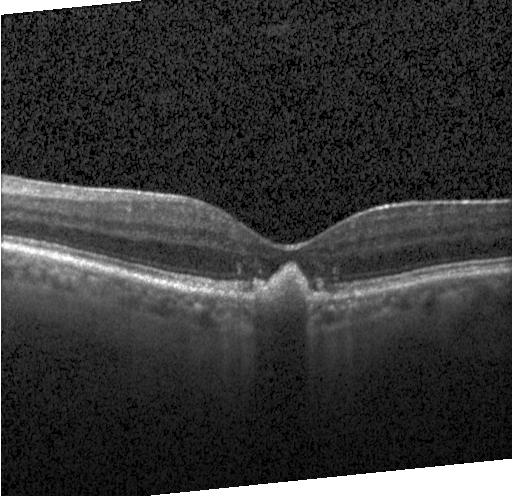

OCT B-scan showing a choroidal neovascular membrane.